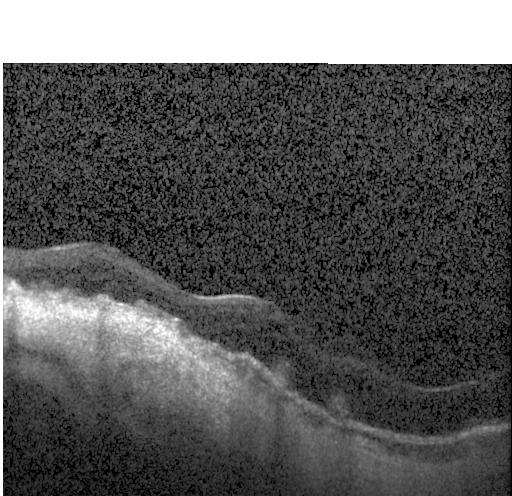

Spectral-domain OCT; retinal OCT cross-section.
OCT finding: choroidal neovascularization.